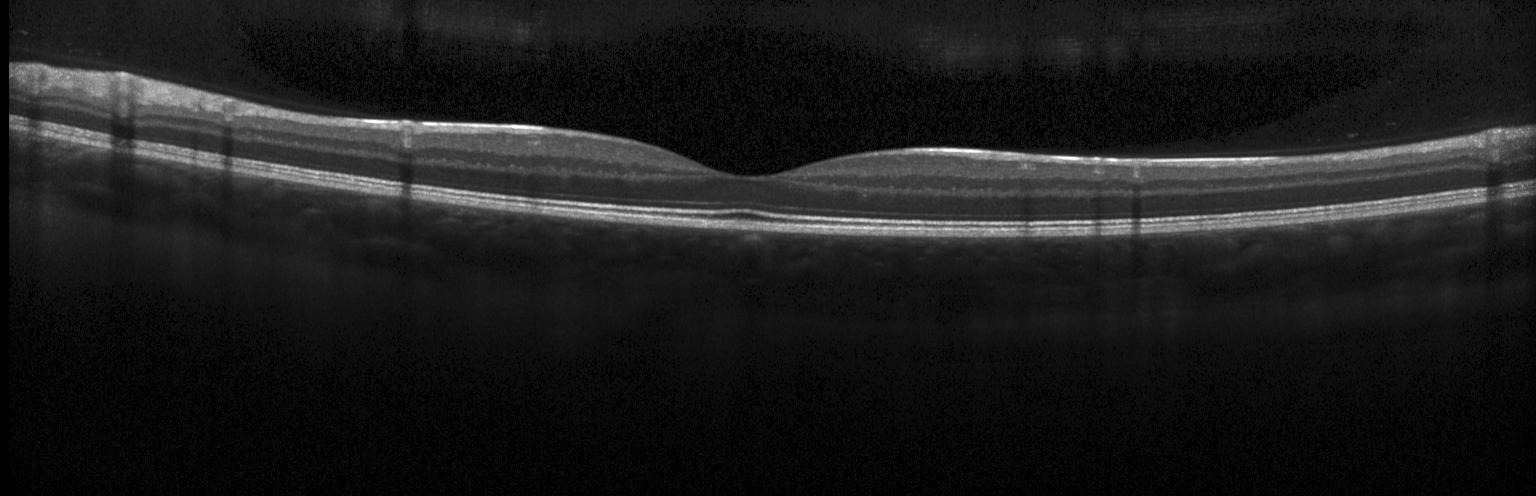 Optical coherence tomography B-scan. Finding: no evidence of CNV, DME, or drusen.